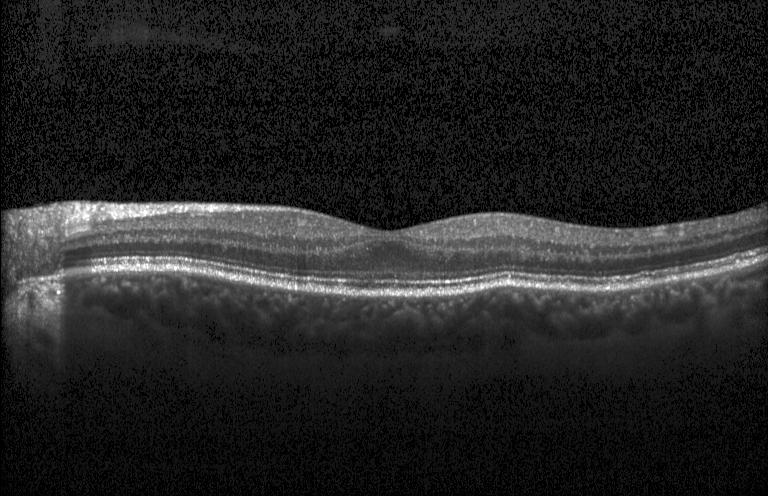
Horizontal scan through the fovea, optical coherence tomography B-scan
The scan shows no CNV, DME, or drusen.